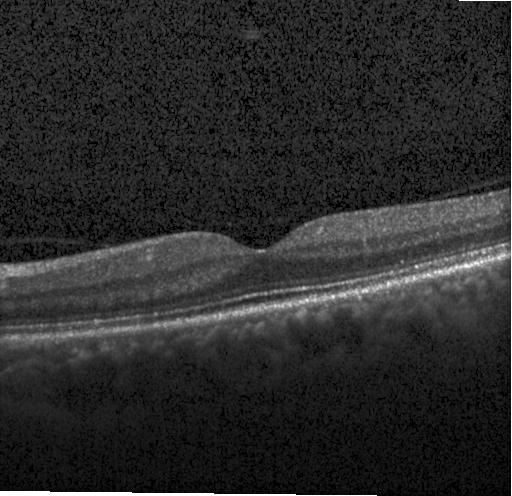
Assessment: no evidence of CNV, DME, or drusen.